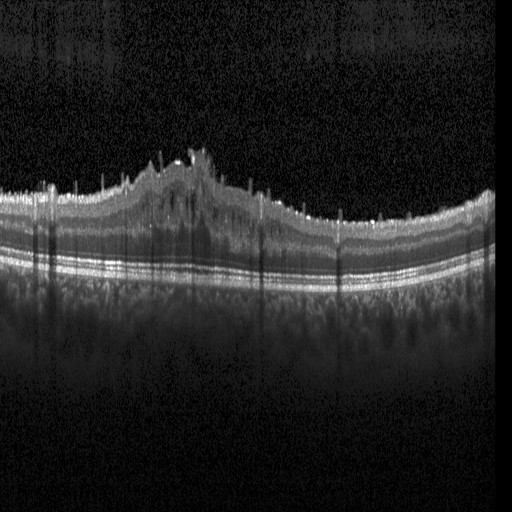 Fovea-centered; spectral-domain optical coherence tomography; OCT B-scan; instrument: Heidelberg Spectralis. Assessment: diabetic macular edema (DME).